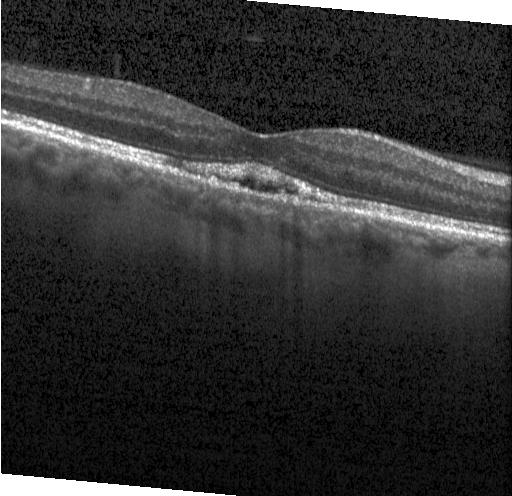 OCT line scan. Heidelberg Spectralis OCT system. Macular scan. Finding: choroidal neovascularization.